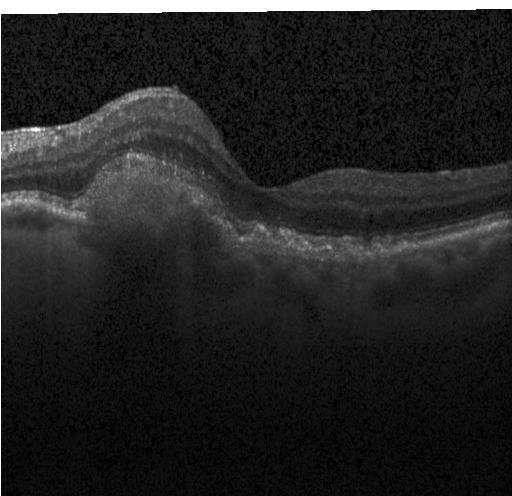

OCT B-scan. Spectral-domain OCT — This B-scan demonstrates choroidal neovascularization.